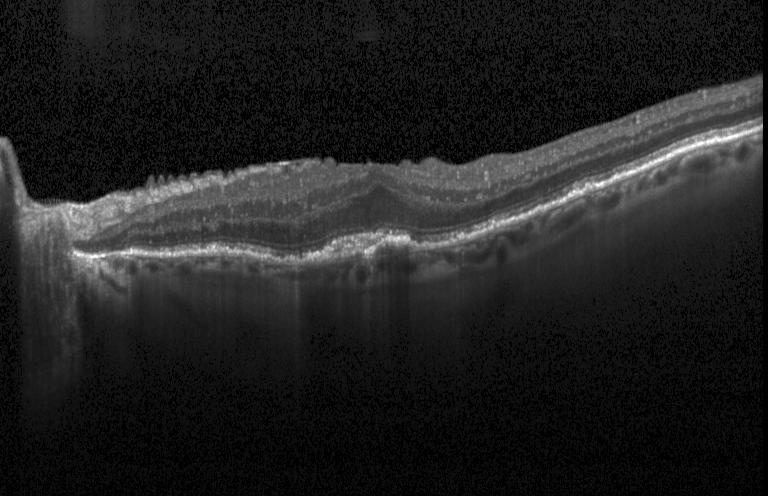 Spectral-domain OCT, Heidelberg Spectralis, optical coherence tomography scan, fovea-centered
OCT finding: a choroidal neovascular membrane.